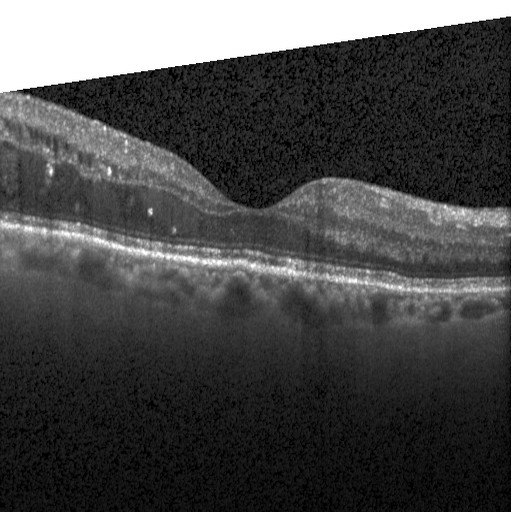
Acquired on a Heidelberg Spectralis · OCT line scan
Finding: DME.